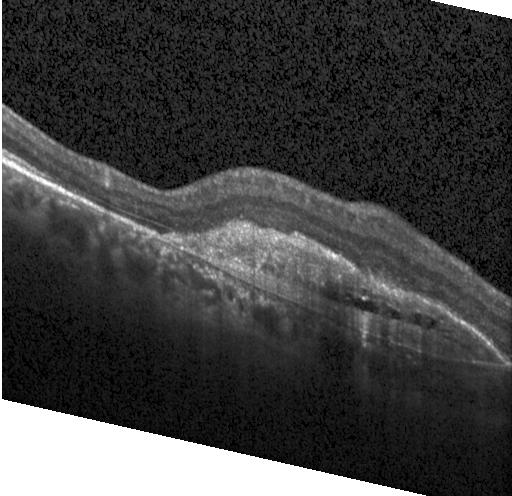 Instrument: Heidelberg Spectralis, spectral-domain optical coherence tomography, optical coherence tomography scan, horizontal scan through the fovea
Dx: a choroidal neovascular membrane.